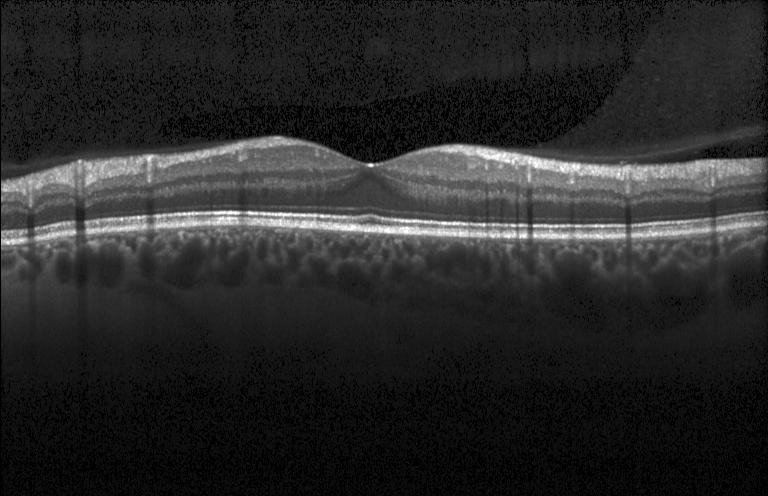

OCT B-scan showing neither CNV, DME, nor drusen.